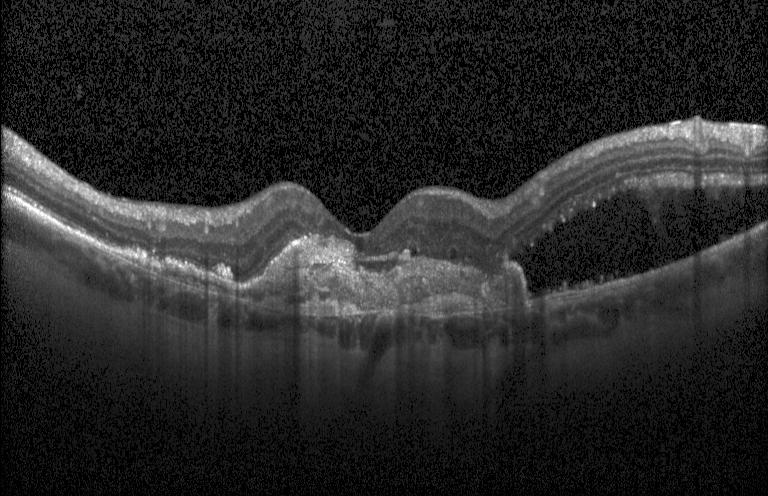 Macular OCT: a choroidal neovascular membrane.